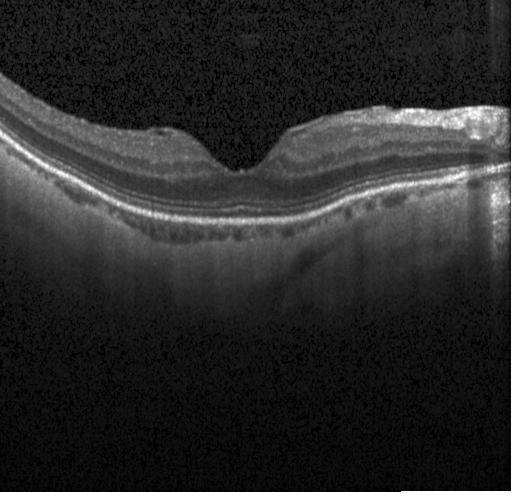 OCT scan showing no evidence of choroidal neovascularization, diabetic macular edema, or drusen.